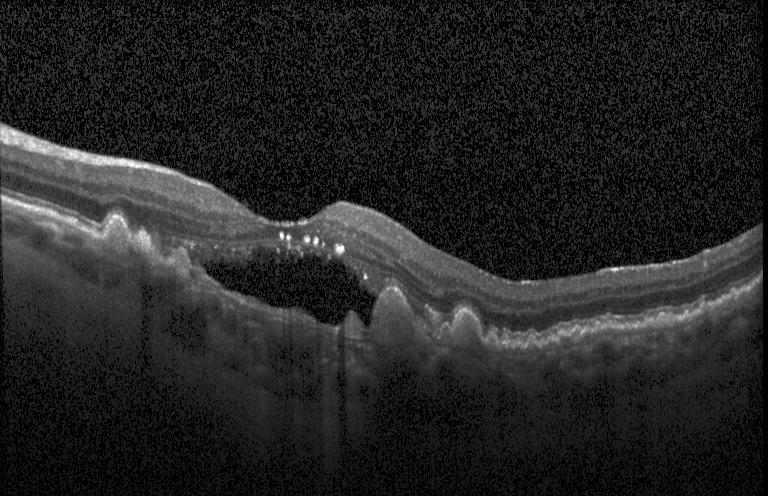 Dx: a choroidal neovascular membrane.